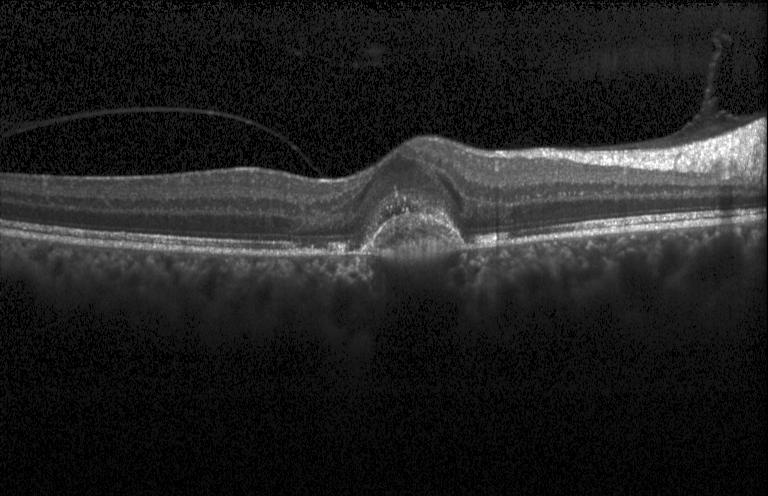
Acquired on a Heidelberg Spectralis. OCT B-scan
Impression: choroidal neovascularization (CNV).